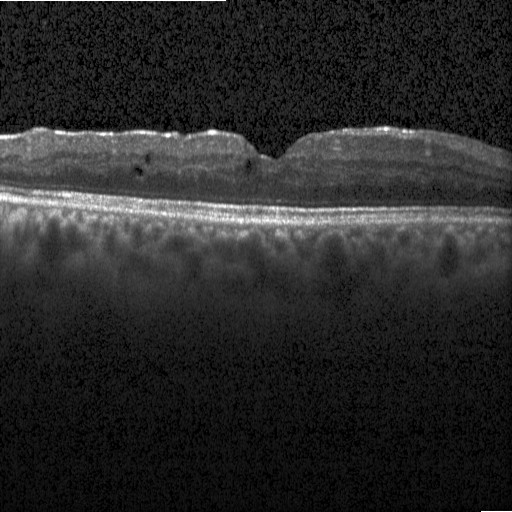

Macular OCT demonstrating diabetic macular edema (DME).